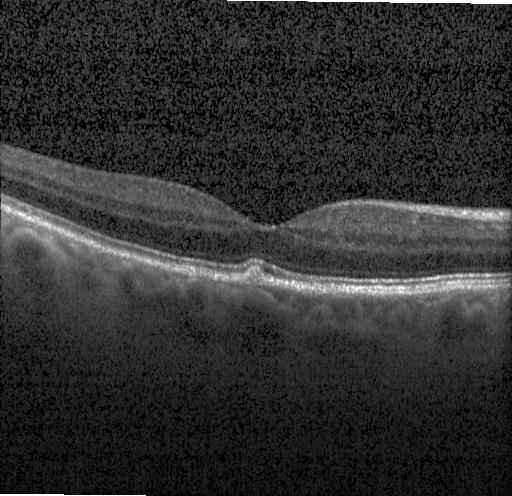
The scan shows multiple drusen.